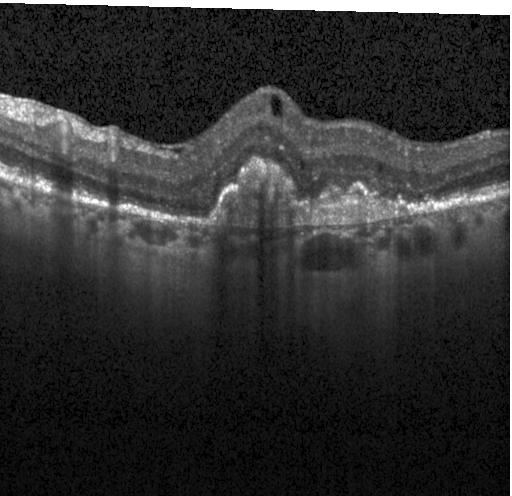

Spectral-domain optical coherence tomography, OCT B-scan, instrument: Heidelberg Spectralis
Diagnosis: CNV.